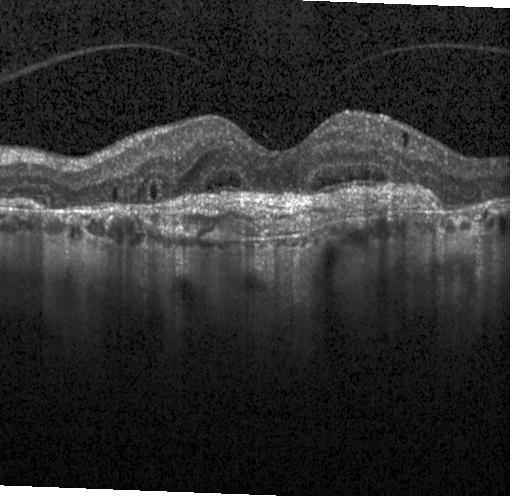 Retinal OCT B-scan.
Diagnosis: a choroidal neovascular membrane.